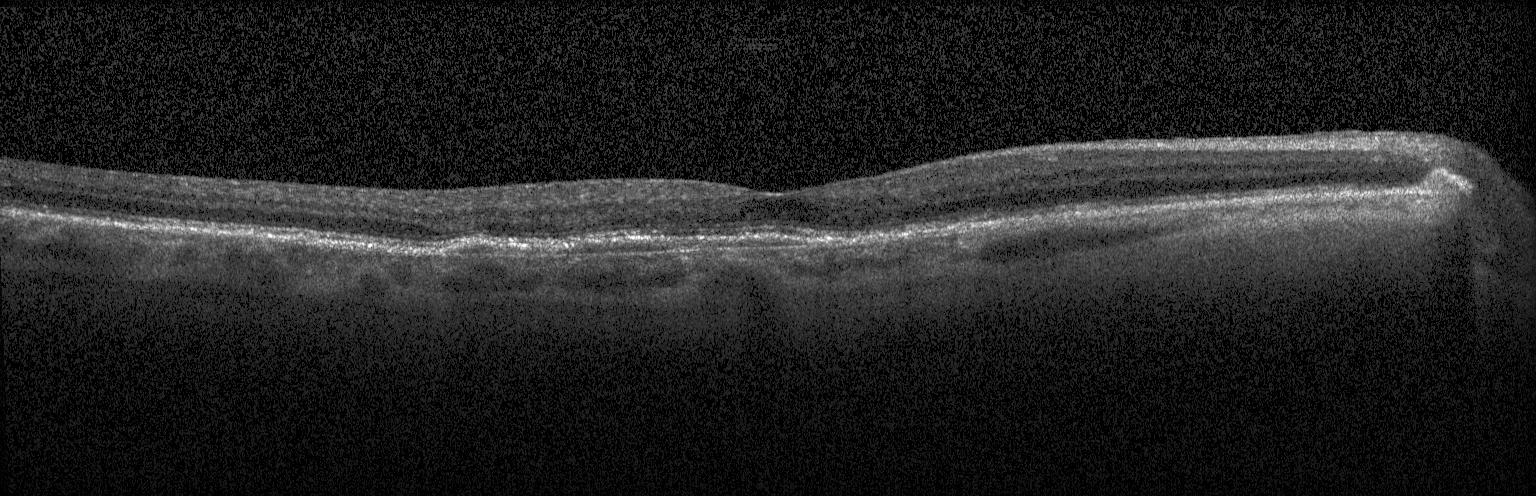 Fovea-centered · spectral-domain optical coherence tomography · retinal OCT cross-section — This B-scan demonstrates CNV.